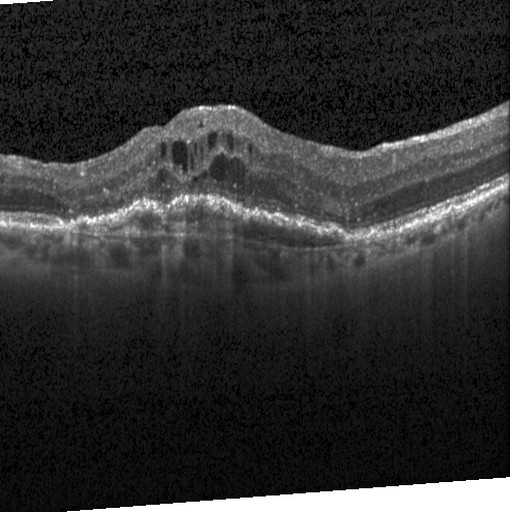
Spectral-domain OCT · optical coherence tomography scan
This B-scan demonstrates diabetic macular edema.